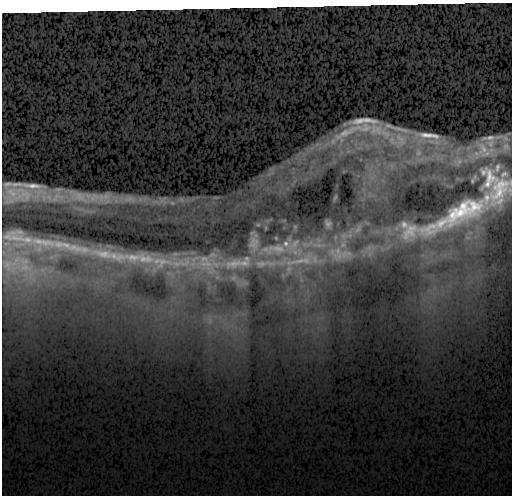

Macular OCT demonstrating a choroidal neovascular membrane.